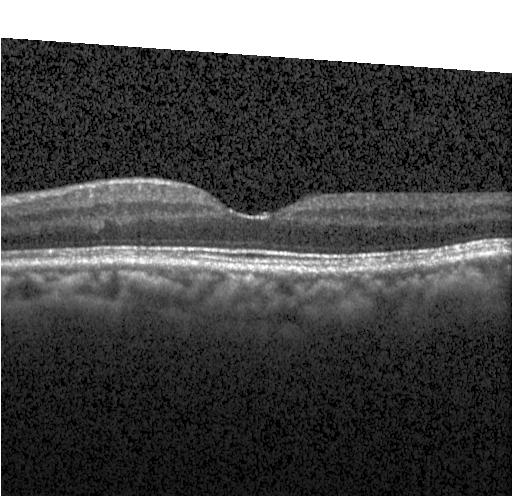
Instrument: Heidelberg Spectralis; optical coherence tomography scan; macular scan — Impression: neither choroidal neovascularization, diabetic macular edema, nor drusen.